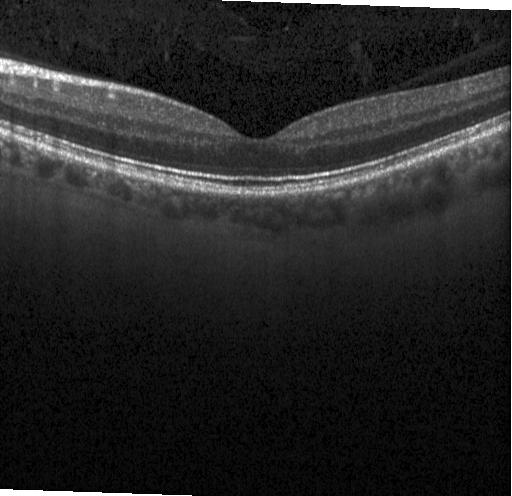
Optical coherence tomography scan — Macular OCT: no CNV, no DME, and no drusen.